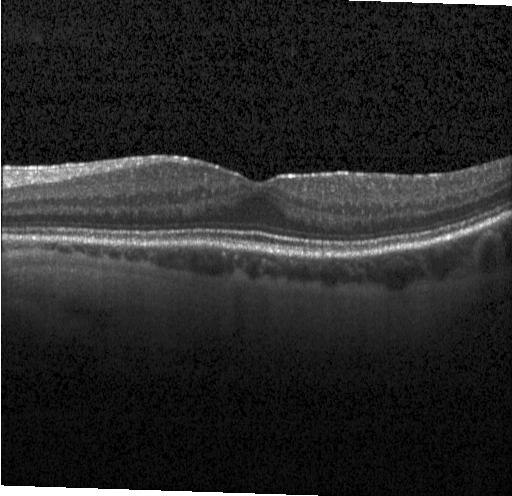 Diagnosis: no CNV, DME, or drusen.